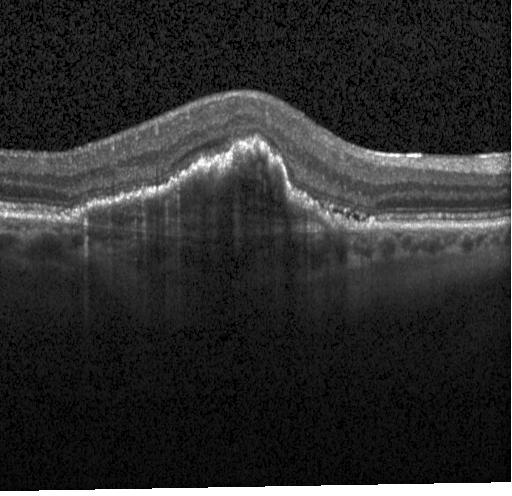
Instrument: Heidelberg Spectralis, retinal OCT B-scan.
Assessment: a choroidal neovascular membrane.